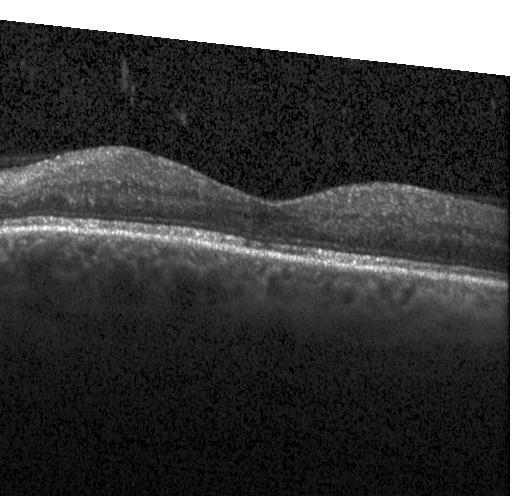

Impression: no choroidal neovascularization, diabetic macular edema, or drusen.